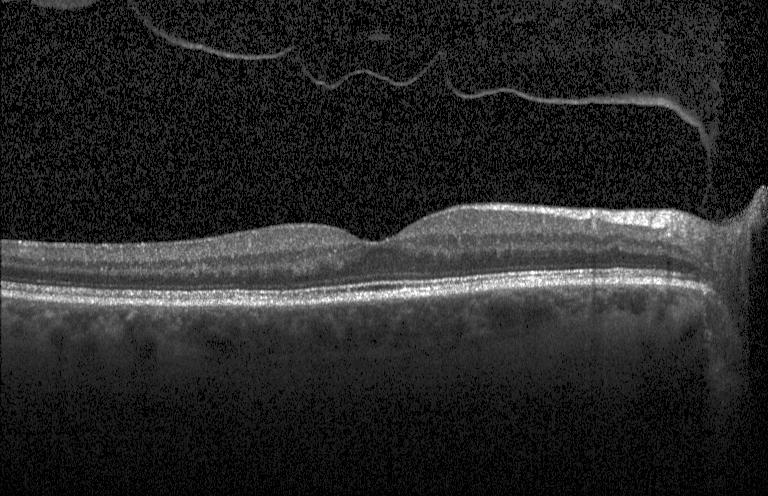
OCT B-scan · Heidelberg Spectralis OCT system · through the macula · SD-OCT
The scan shows no CNV, DME, or drusen.